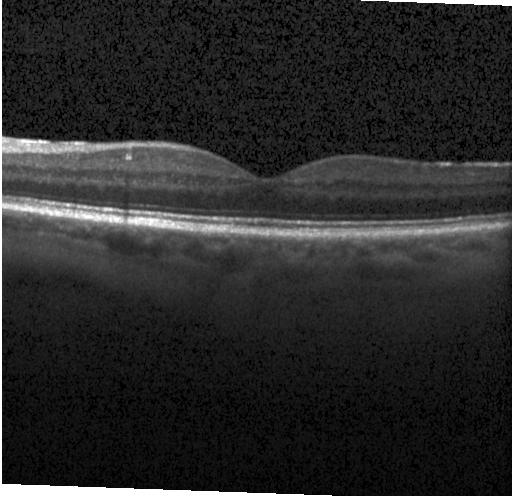
Optical coherence tomography B-scan · centered on the fovea · SD-OCT — Impression: no evidence of choroidal neovascularization, diabetic macular edema, or drusen.